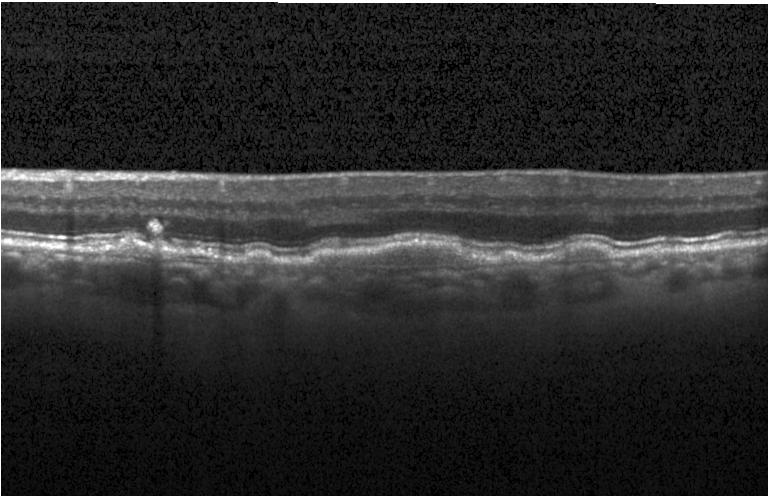 Spectral-domain OCT; optical coherence tomography scan; fovea-centered; Heidelberg Spectralis OCT system
Drusen.